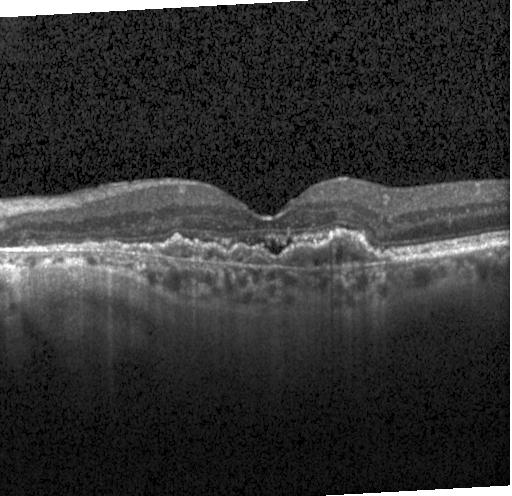
Diagnosis: a choroidal neovascular membrane.